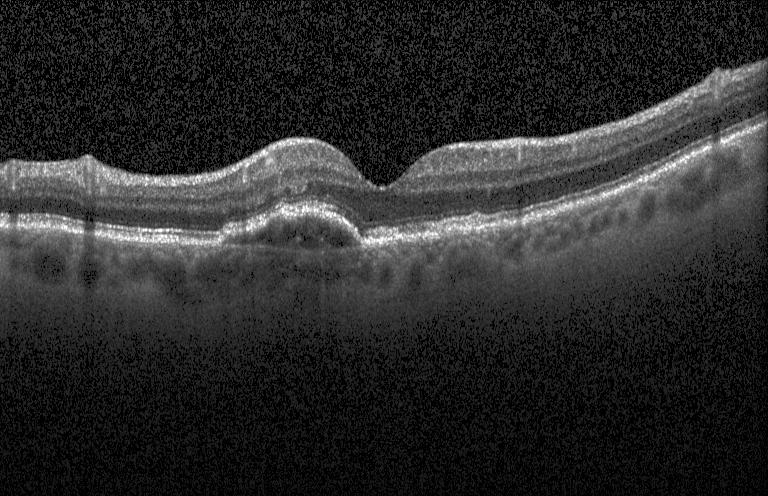
Macular scan; instrument: Heidelberg Spectralis; SD-OCT; optical coherence tomography scan
Diagnosis: a choroidal neovascular membrane.